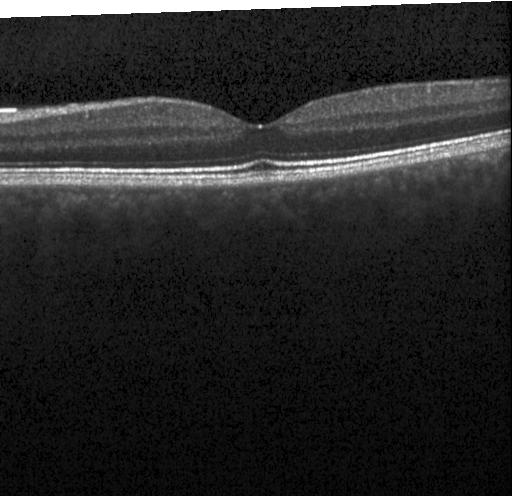 Spectral-domain OCT; optical coherence tomography B-scan.
This B-scan demonstrates no choroidal neovascularization, no diabetic macular edema, and no drusen.